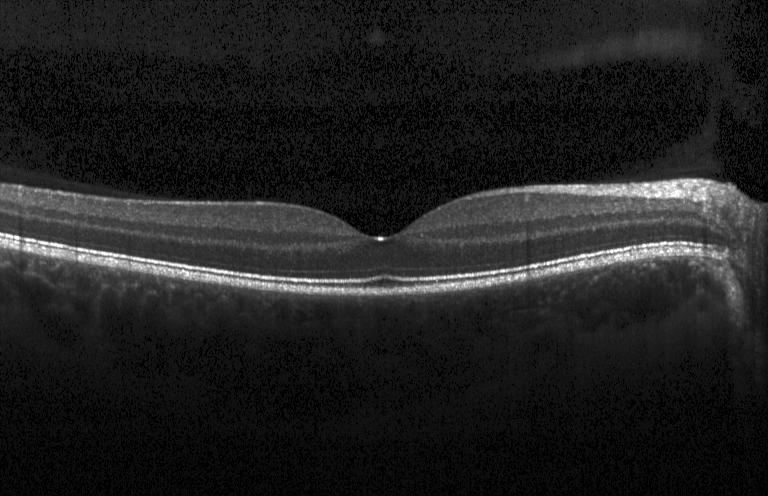 SD-OCT · through the macula · OCT line scan · Heidelberg Spectralis OCT system.
Impression: no choroidal neovascularization, no diabetic macular edema, and no drusen.